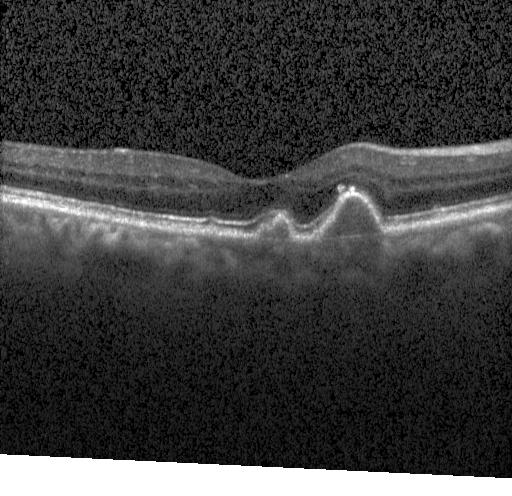
OCT B-scan, SD-OCT. Diagnosis: sub-RPE drusenoid deposits.